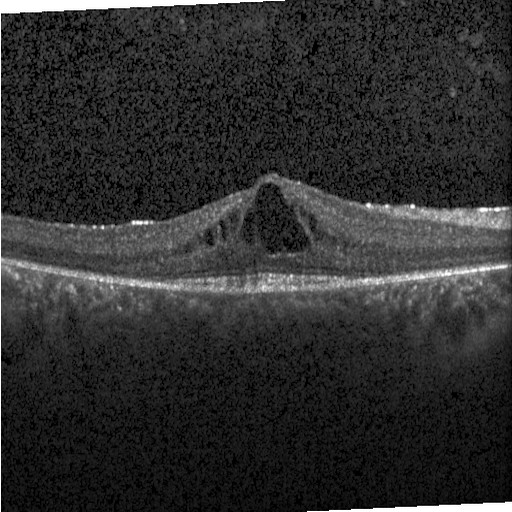 Retinal OCT B-scan — DME.